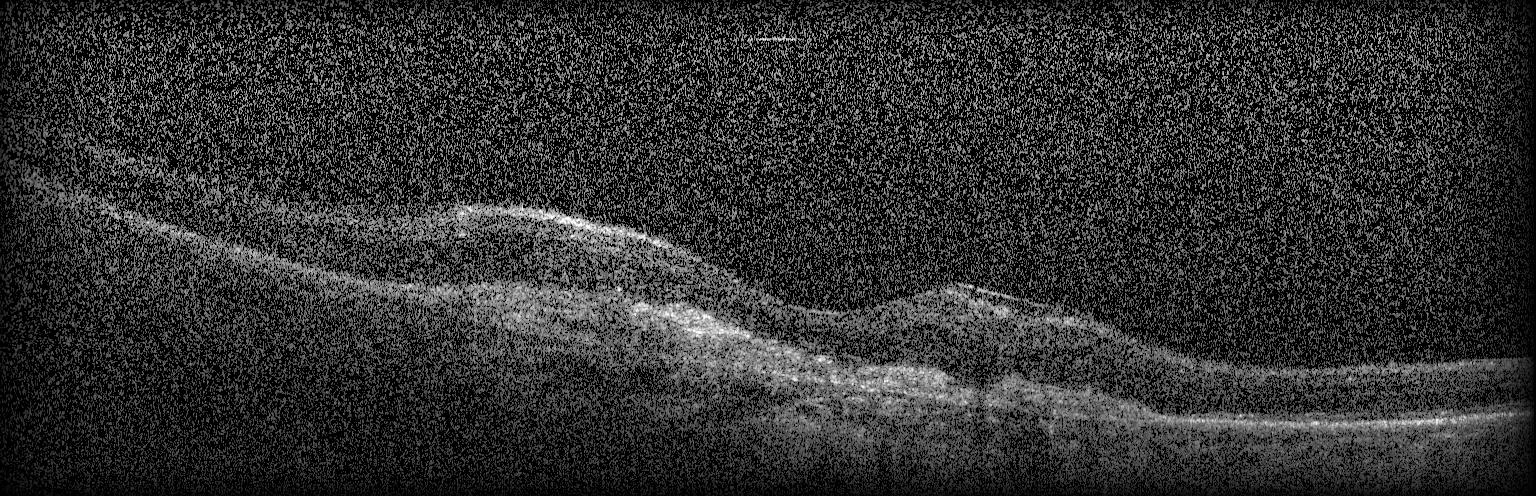
Spectral-domain OCT B-scan: choroidal neovascularization (CNV).